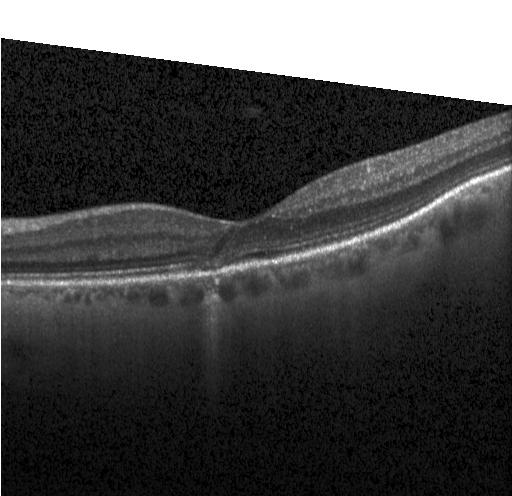 Spectral-domain optical coherence tomography, Heidelberg Spectralis, OCT line scan.
Diagnosis: no choroidal neovascularization, diabetic macular edema, or drusen.